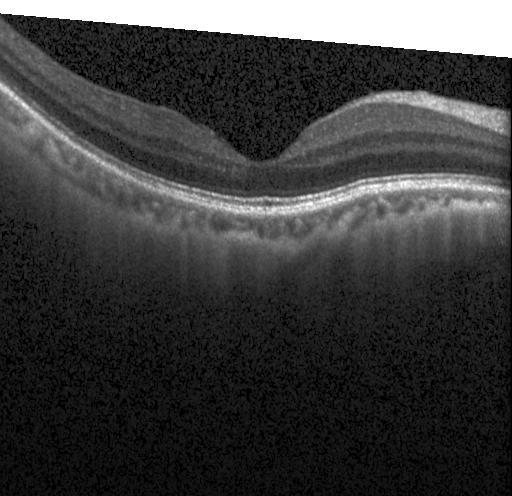 The scan shows no CNV, DME, or drusen.